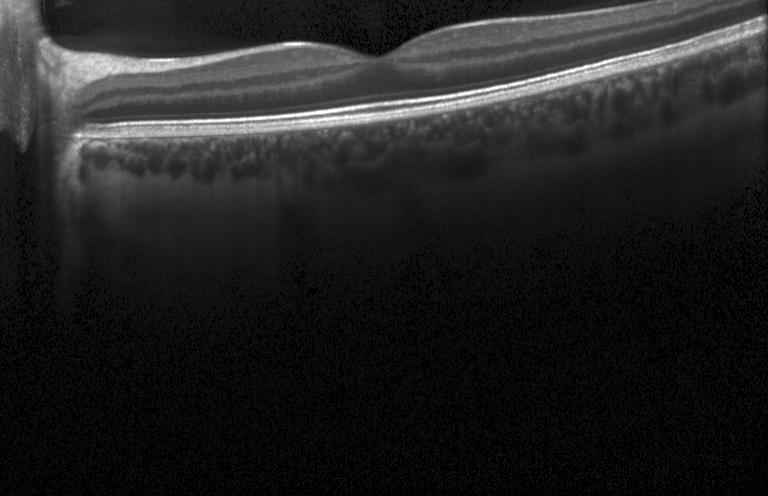 Optical coherence tomography B-scan.
Diagnosis: neither choroidal neovascularization, diabetic macular edema, nor drusen.